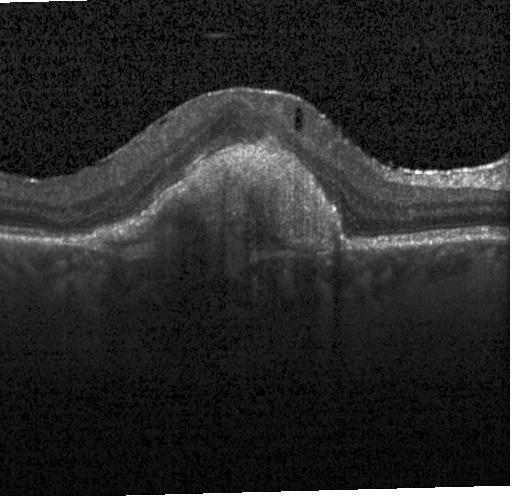 Retinal OCT B-scan. Through the macula. SD-OCT. Heidelberg Spectralis OCT system — Impression: choroidal neovascularization.